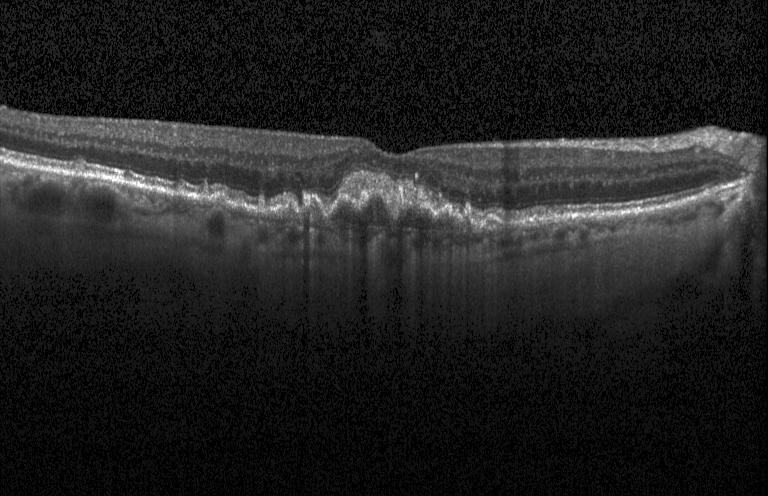 Retinal OCT B-scan — Dx: CNV.